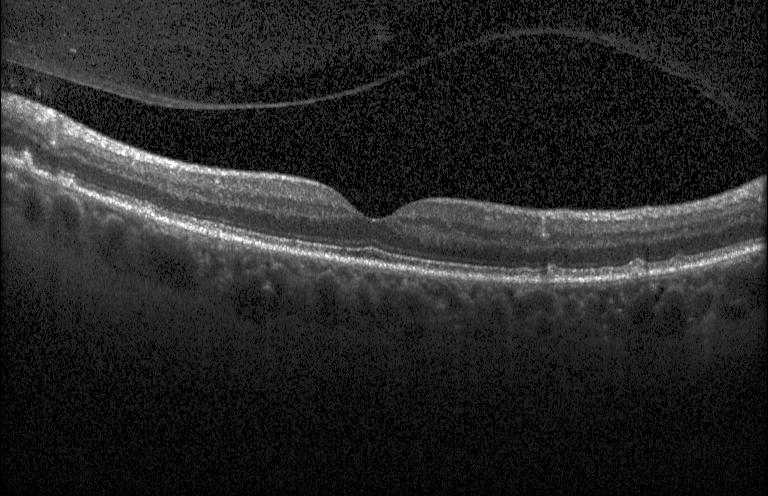
Spectral-domain OCT B-scan: no evidence of CNV, DME, or drusen.